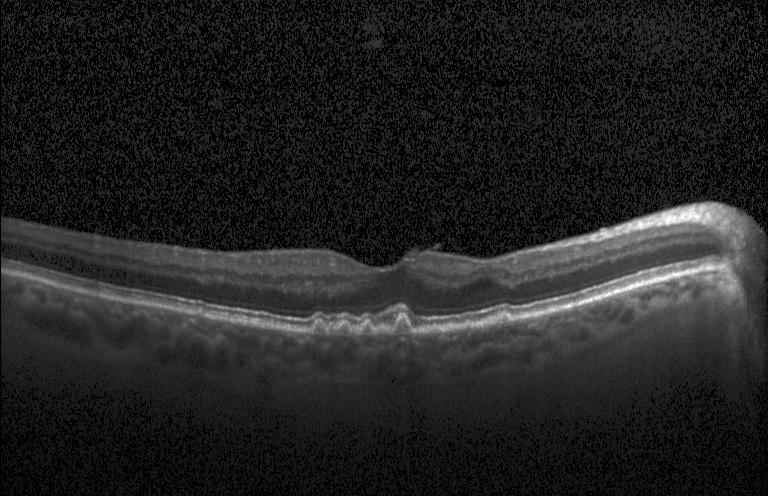
OCT B-scan.
Diagnosis: sub-RPE drusenoid deposits.